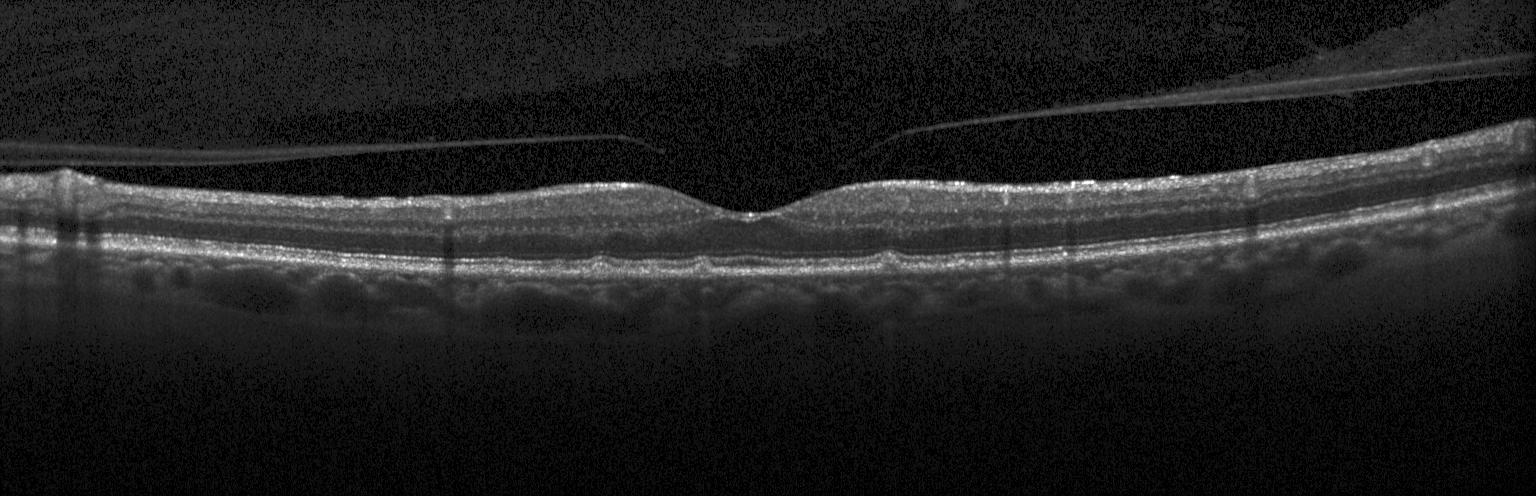
OCT line scan — Assessment: multiple drusen.